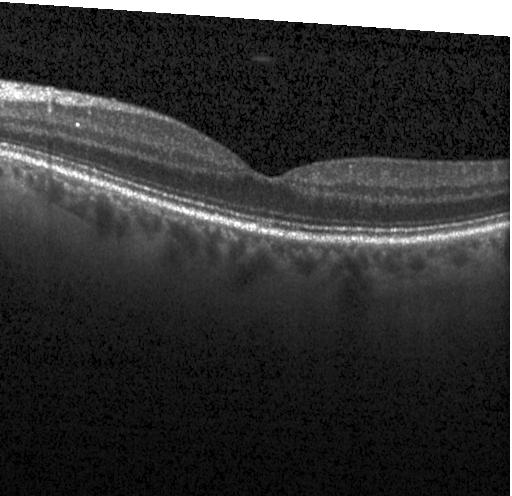
Diagnosis: neither choroidal neovascularization, diabetic macular edema, nor drusen.